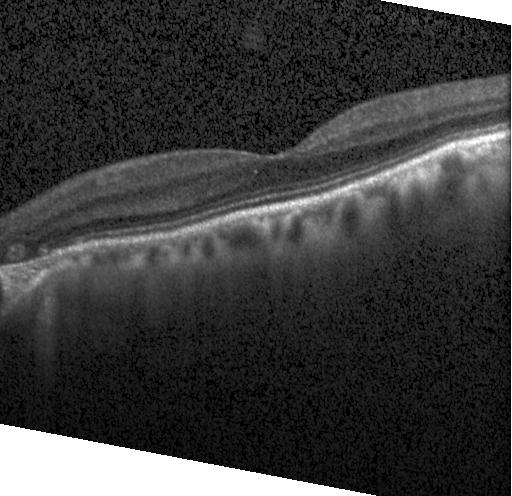

Fovea-centered. Optical coherence tomography B-scan.
Finding: no CNV, DME, or drusen.